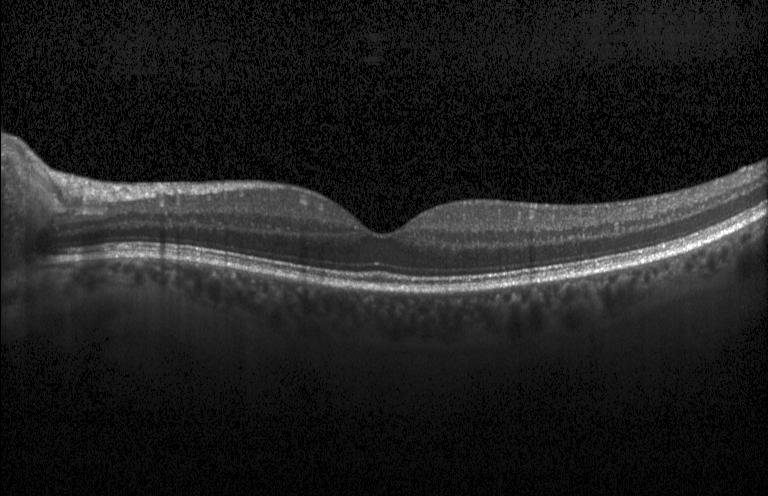

Diagnosis: no CNV, no DME, and no drusen.